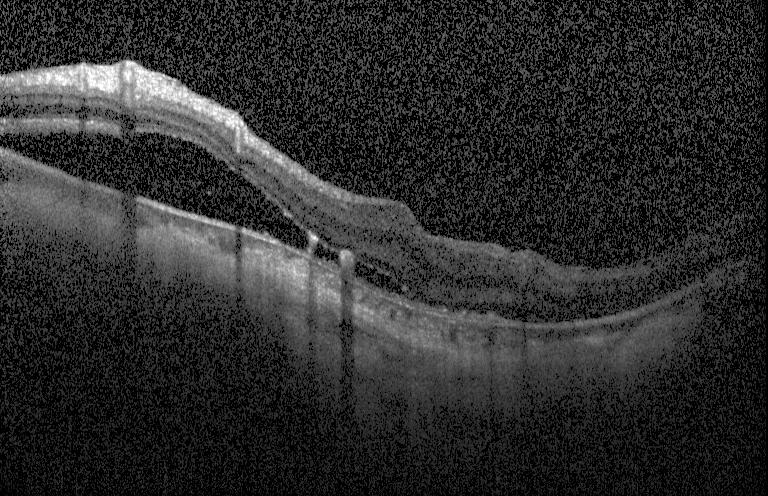
OCT B-scan; through the macula; SD-OCT; Heidelberg Spectralis OCT system — Diagnosis: a choroidal neovascular membrane.